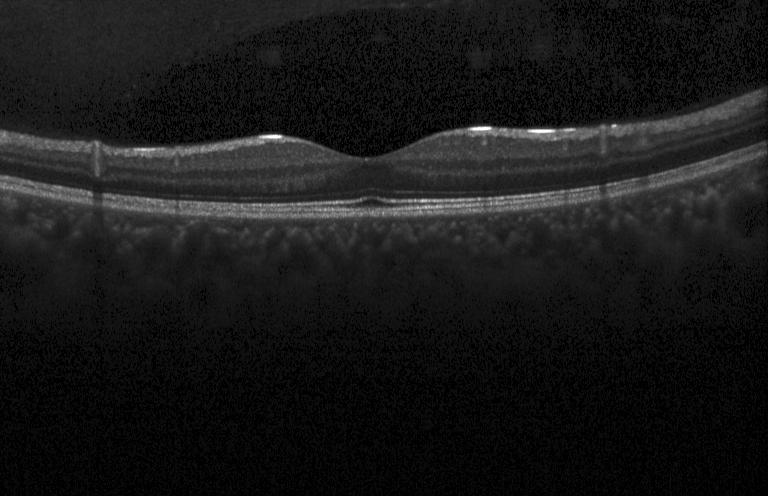 OCT B-scan — Dx: no evidence of choroidal neovascularization, diabetic macular edema, or drusen.